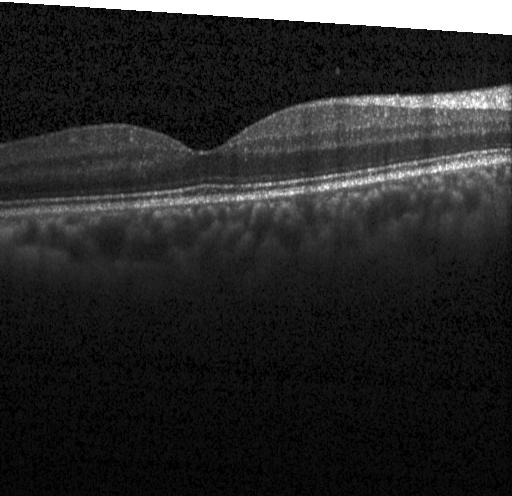 Dx: no choroidal neovascularization, diabetic macular edema, or drusen.